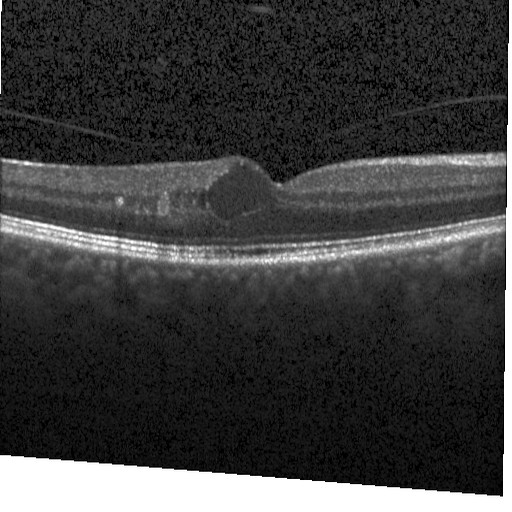

SD-OCT. Heidelberg Spectralis OCT system. Fovea-centered. OCT B-scan. Assessment: diabetic macular edema.